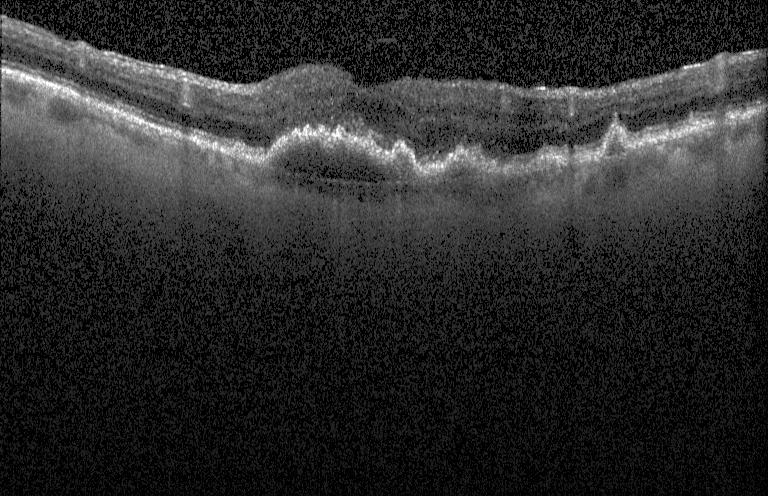 Macular OCT: choroidal neovascularization (CNV).